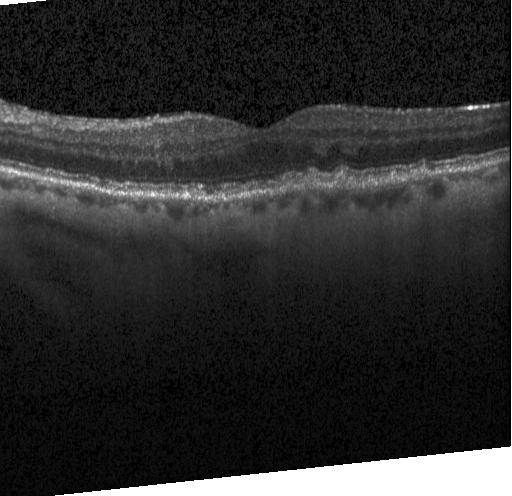

Macular OCT demonstrating drusen.